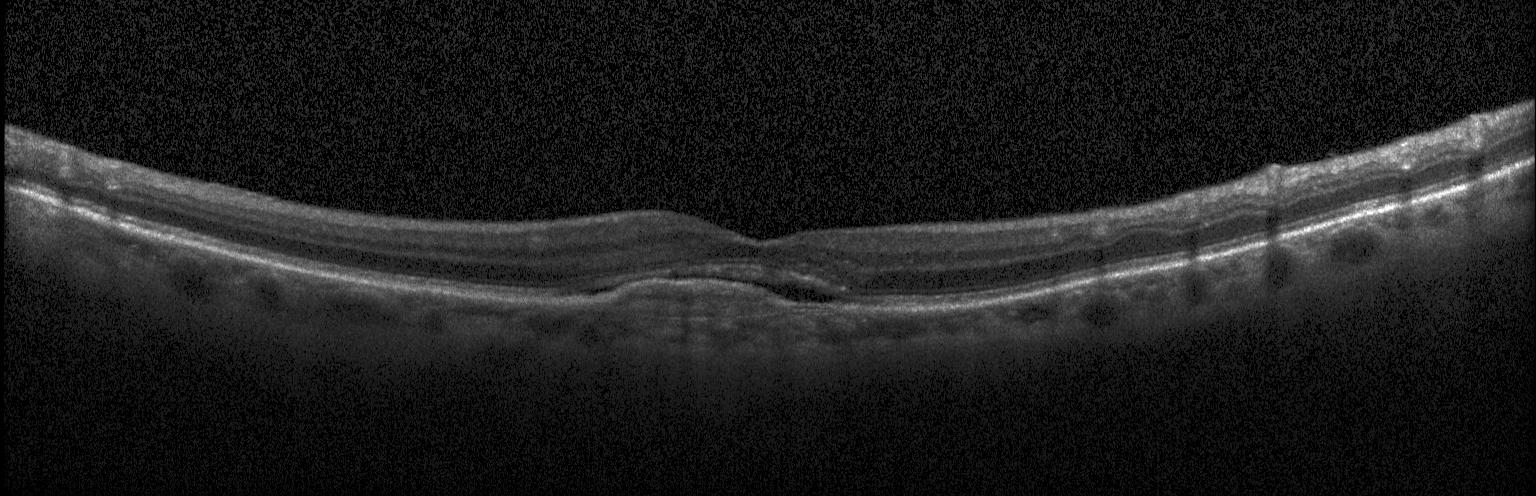

This B-scan demonstrates a choroidal neovascular membrane.